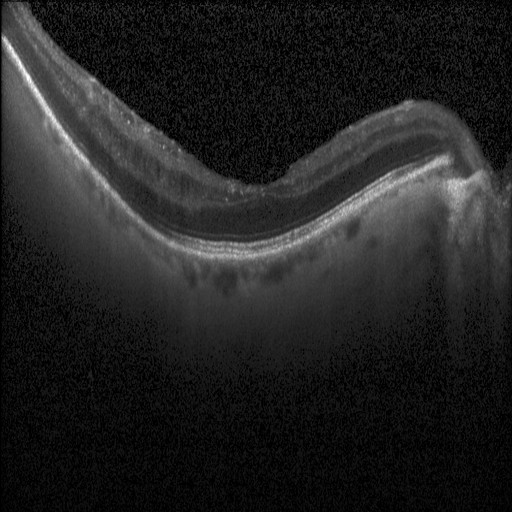
Optical coherence tomography scan. Spectral-domain OCT. Macular scan.
Dx: DME.